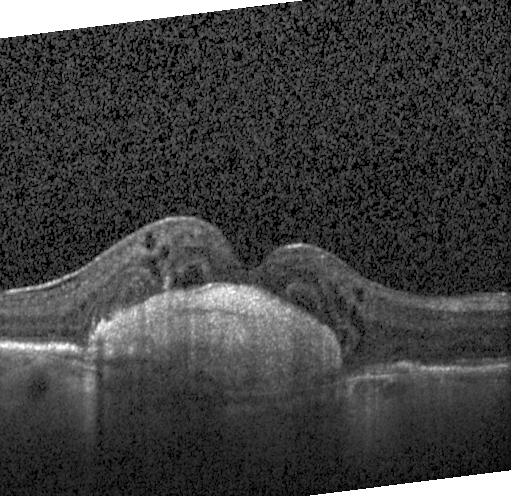

Macular scan · Heidelberg Spectralis · retinal OCT B-scan.
Macular OCT: a choroidal neovascular membrane.